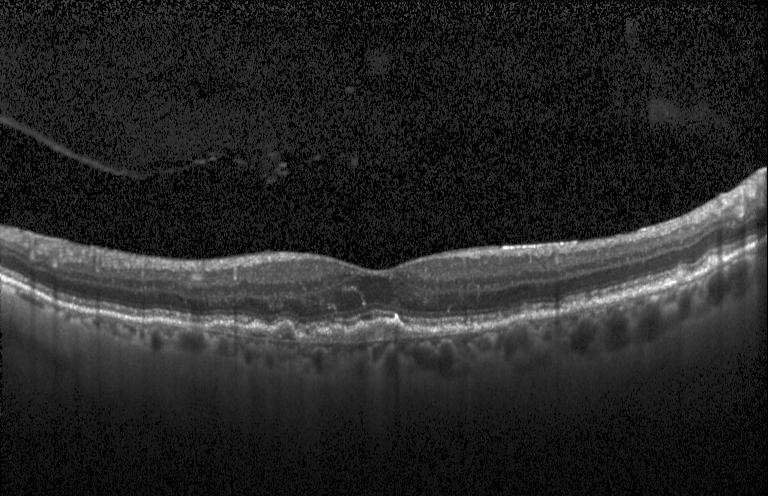

Macular OCT demonstrating a choroidal neovascular membrane.